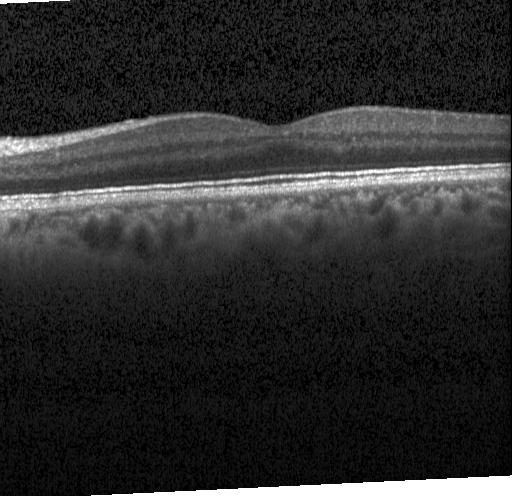 Assessment: no CNV, DME, or drusen.